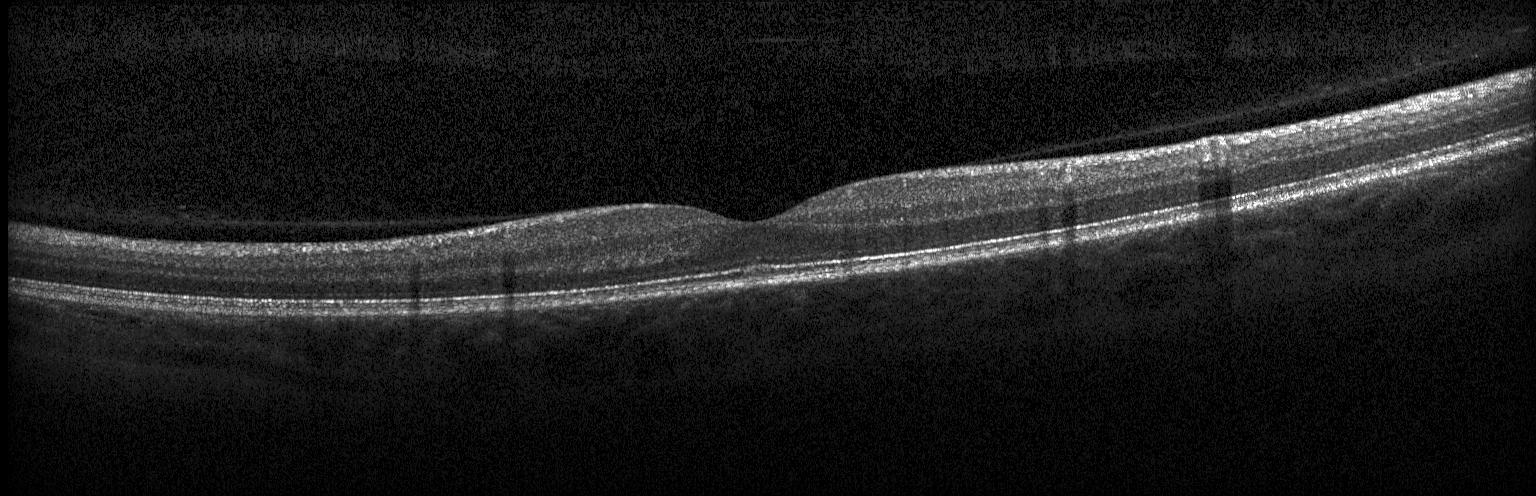 Acquired on a Heidelberg Spectralis. Spectral-domain optical coherence tomography. OCT line scan. Fovea-centered
Diagnosis: neither choroidal neovascularization, diabetic macular edema, nor drusen.